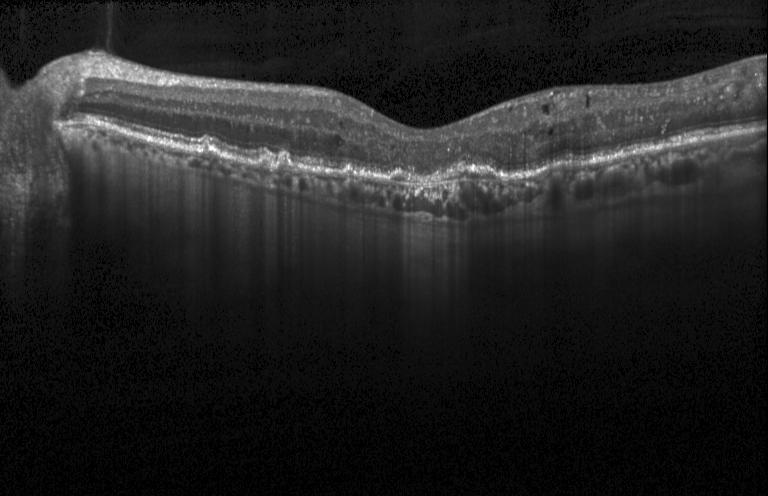
OCT finding: choroidal neovascularization.